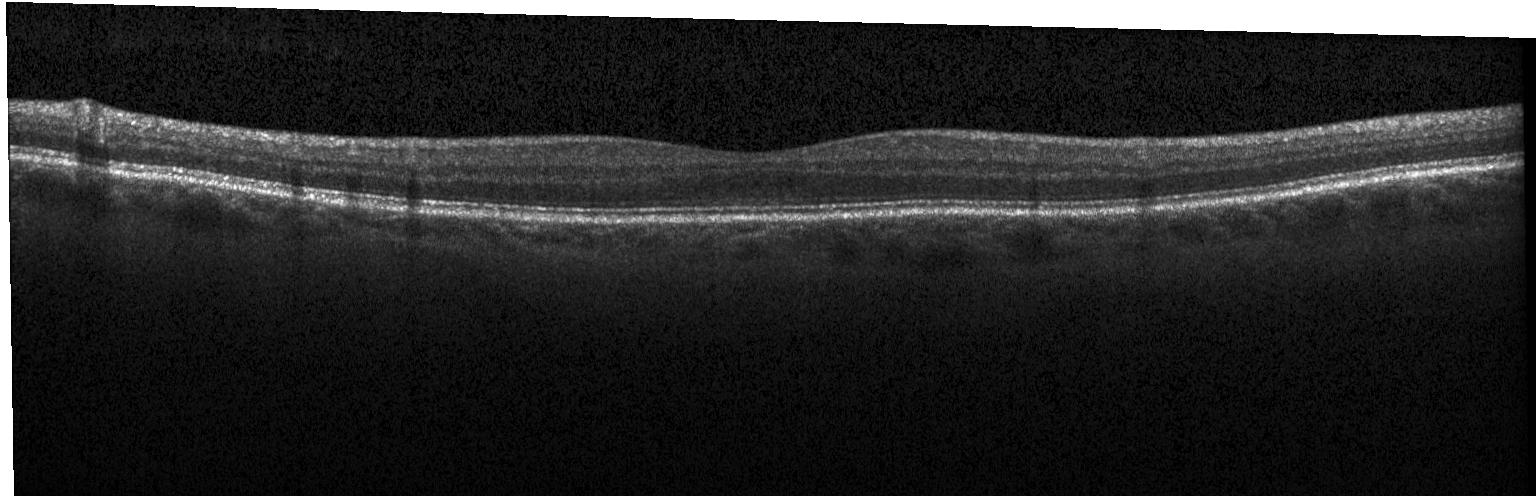

Horizontal scan through the fovea; OCT line scan — Diagnosis: no evidence of choroidal neovascularization, diabetic macular edema, or drusen.